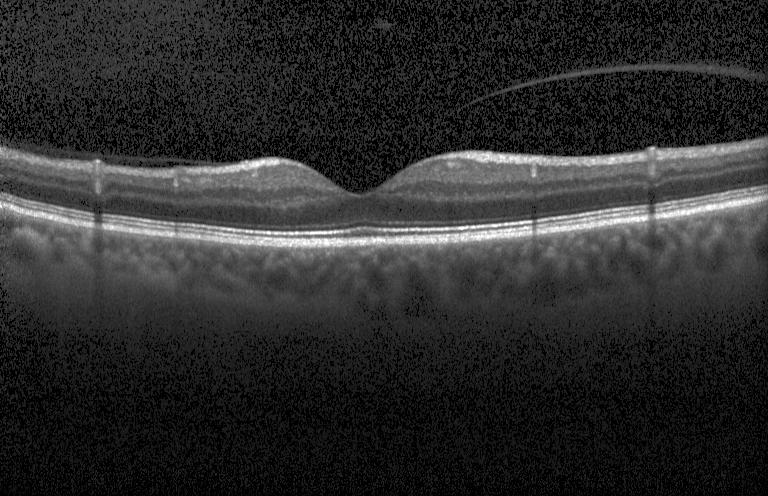 SD-OCT. Retinal OCT B-scan. Through the macula. OCT finding: no CNV, no DME, and no drusen.